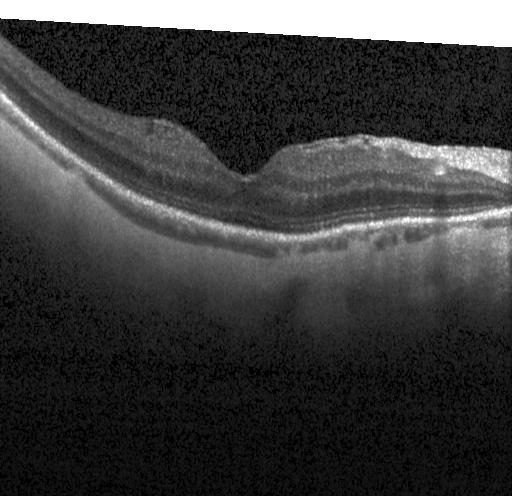 No evidence of choroidal neovascularization, diabetic macular edema, or drusen.